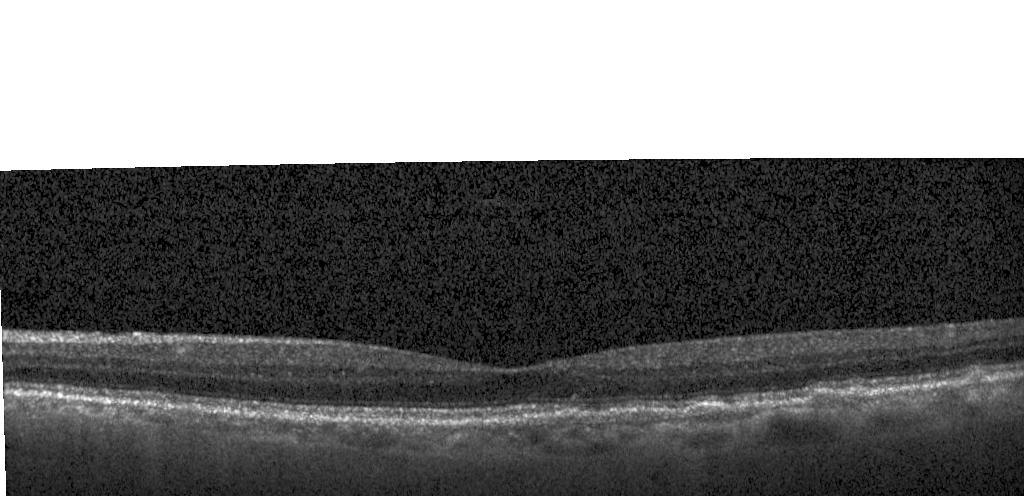

The scan shows sub-RPE drusenoid deposits.